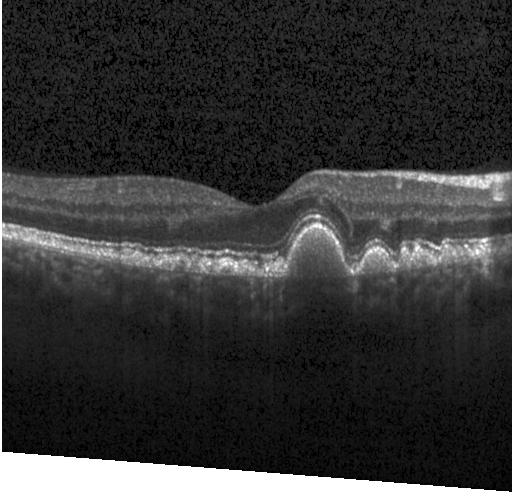

OCT line scan — Finding: multiple drusen.